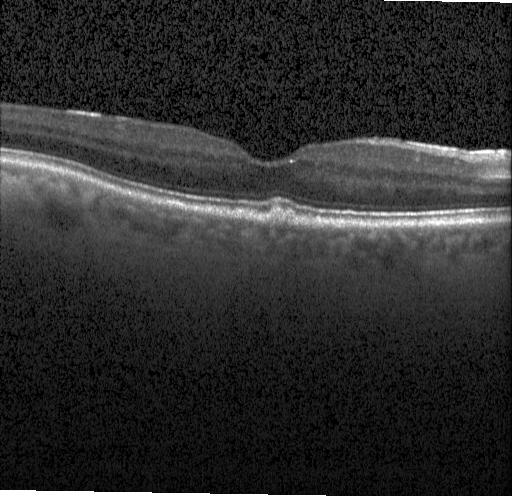

Optical coherence tomography scan.
Diagnosis: sub-RPE drusenoid deposits.